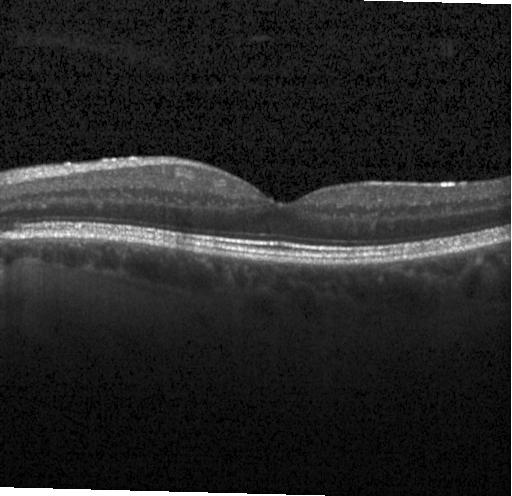 Impression: no choroidal neovascularization, no diabetic macular edema, and no drusen.